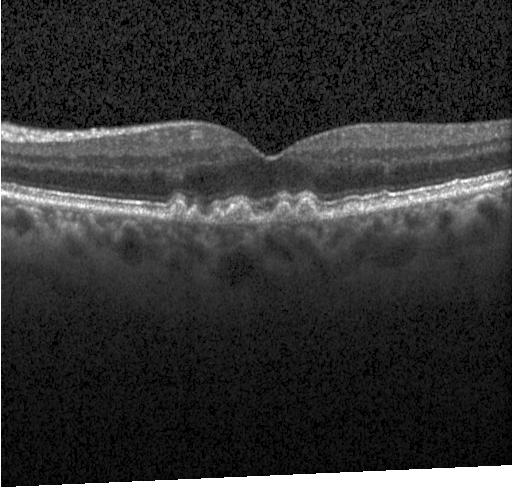 Diagnosis: drusen.